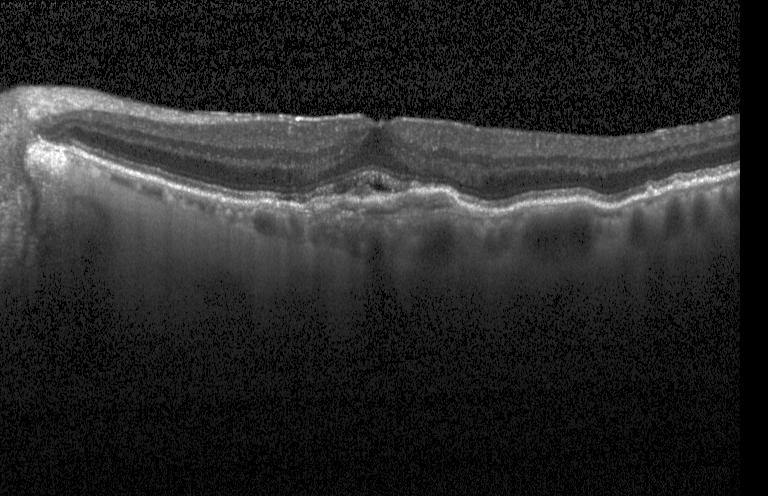 Retinal OCT cross-section — The scan shows a choroidal neovascular membrane.